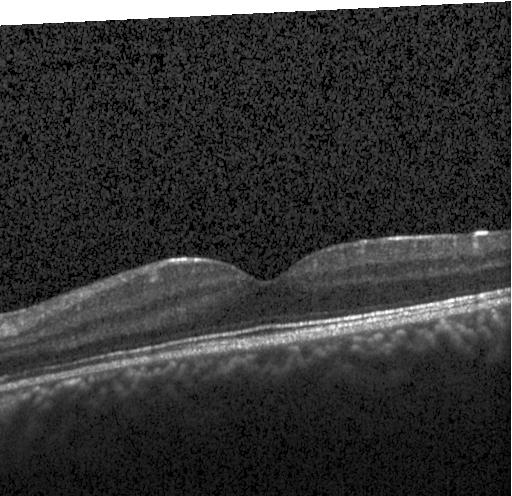

Macular OCT: no CNV, no DME, and no drusen.